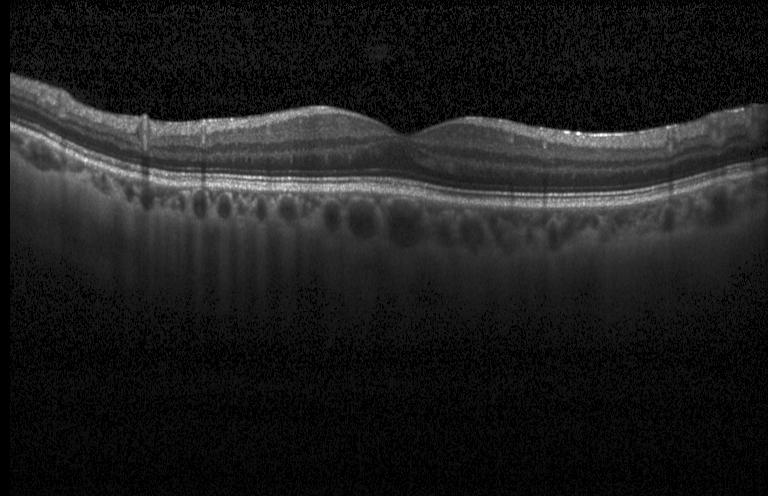

Retinal OCT B-scan. Assessment: no evidence of CNV, DME, or drusen.